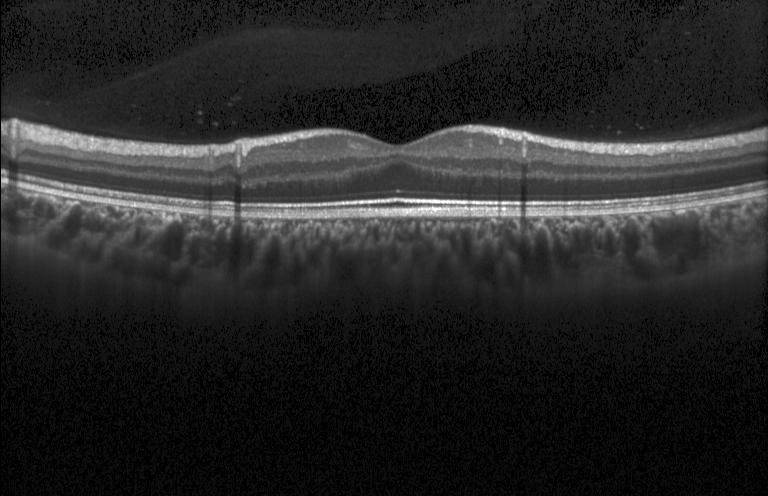 Optical coherence tomography scan, spectral-domain optical coherence tomography — The scan shows neither choroidal neovascularization, diabetic macular edema, nor drusen.